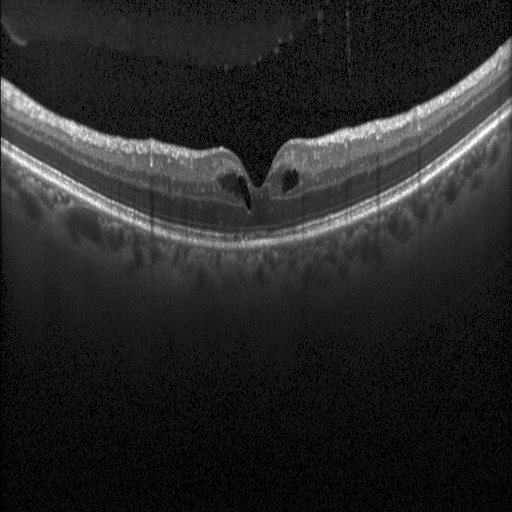
OCT B-scan. This B-scan demonstrates DME.